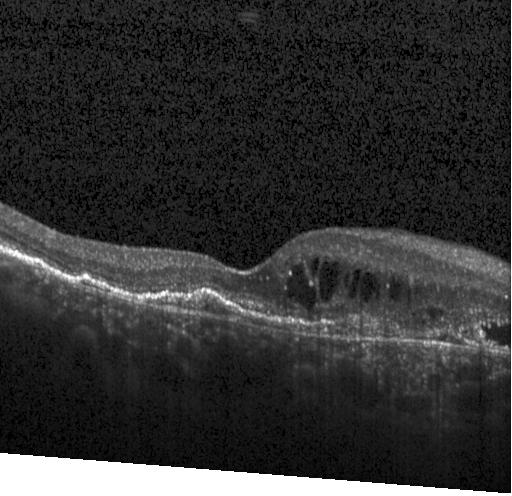

OCT B-scan. OCT finding: CNV.